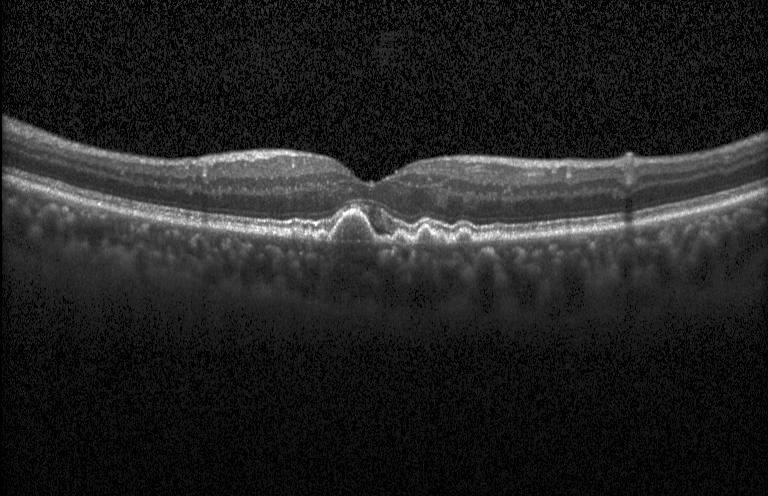

Retinal OCT cross-section; instrument: Heidelberg Spectralis; macular scan
Sub-RPE drusenoid deposits.